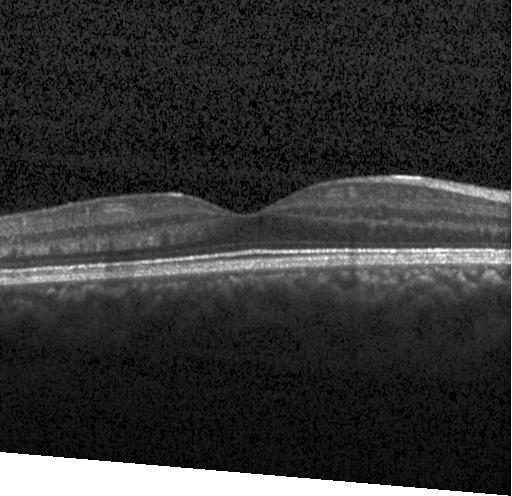

Acquired on a Heidelberg Spectralis, optical coherence tomography scan.
This B-scan demonstrates neither choroidal neovascularization, diabetic macular edema, nor drusen.